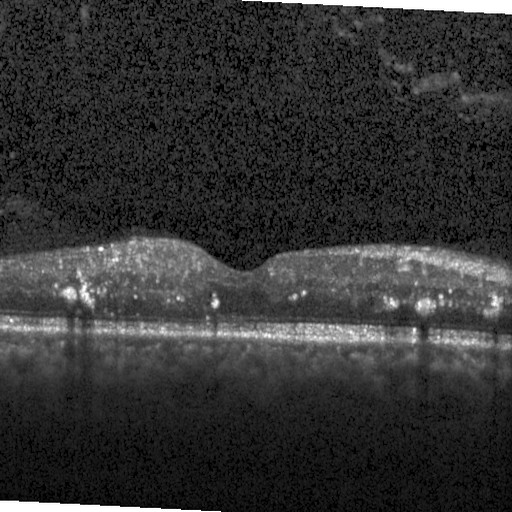
Dx: diabetic macular edema.